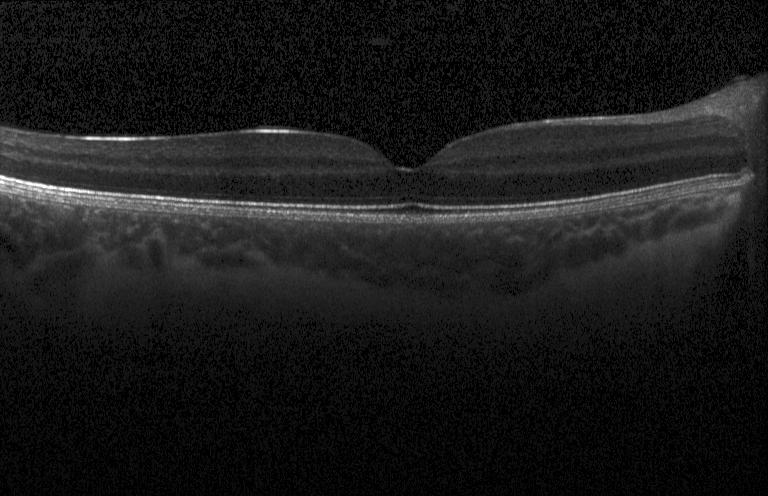 Retinal OCT cross-section · centered on the fovea · Heidelberg Spectralis OCT system.
Assessment: no choroidal neovascularization, diabetic macular edema, or drusen.